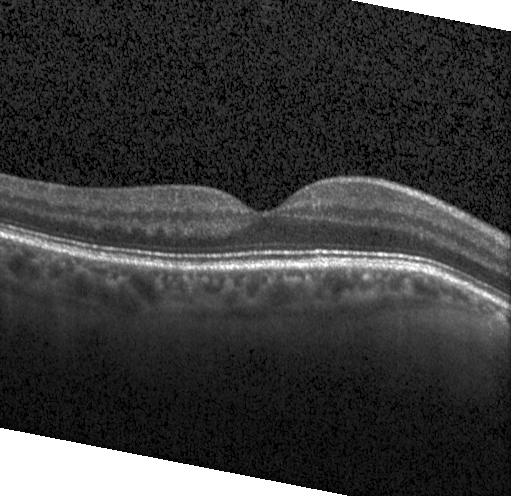

Retinal OCT B-scan. The scan shows no choroidal neovascularization, no diabetic macular edema, and no drusen.